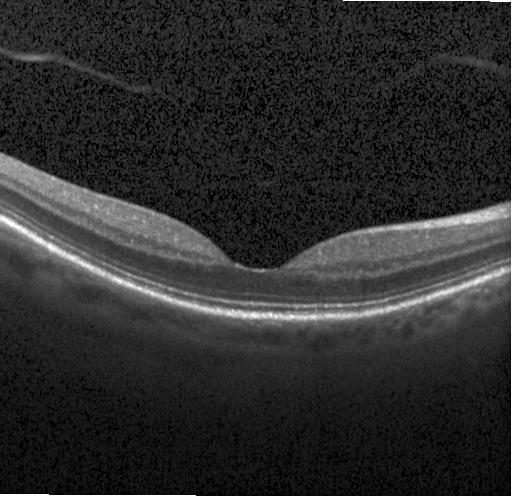 OCT B-scan showing no CNV, no DME, and no drusen.